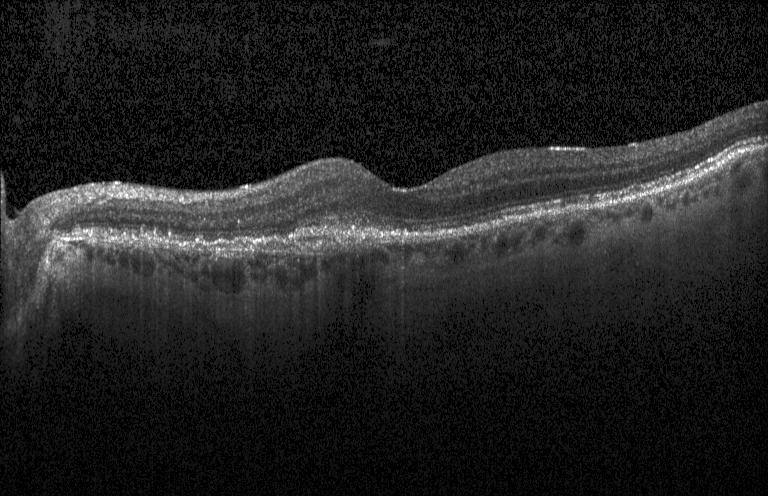 Impression: CNV.